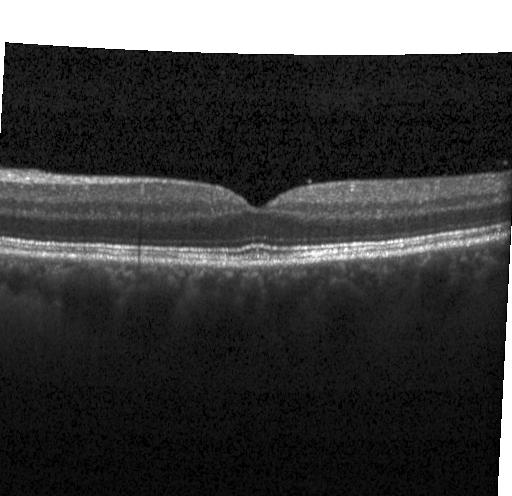
Instrument: Heidelberg Spectralis · optical coherence tomography scan · SD-OCT.
Neither choroidal neovascularization, diabetic macular edema, nor drusen.